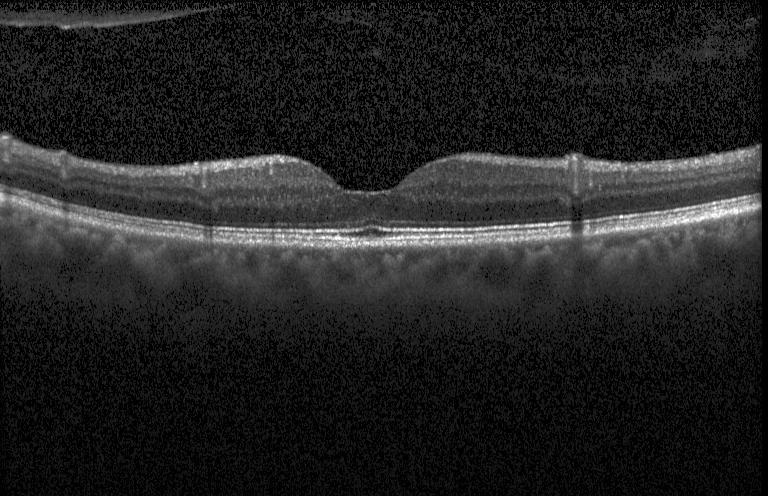

Heidelberg Spectralis. OCT B-scan — Impression: no choroidal neovascularization, diabetic macular edema, or drusen.